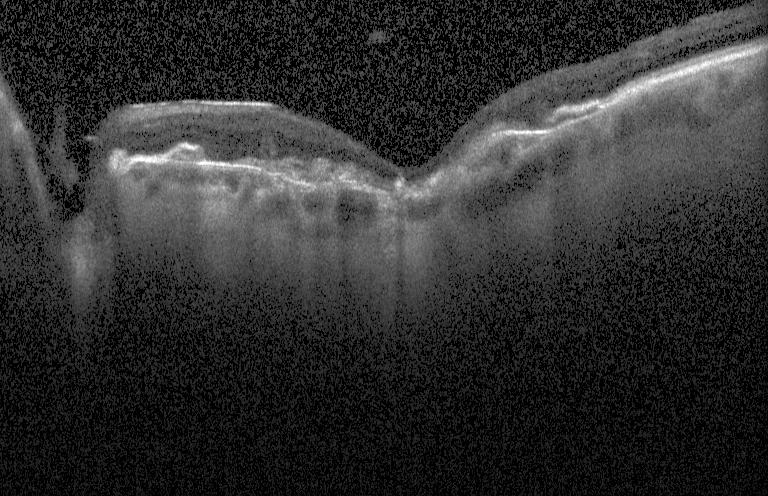 Heidelberg Spectralis OCT system; OCT line scan
Diagnosis: a choroidal neovascular membrane.